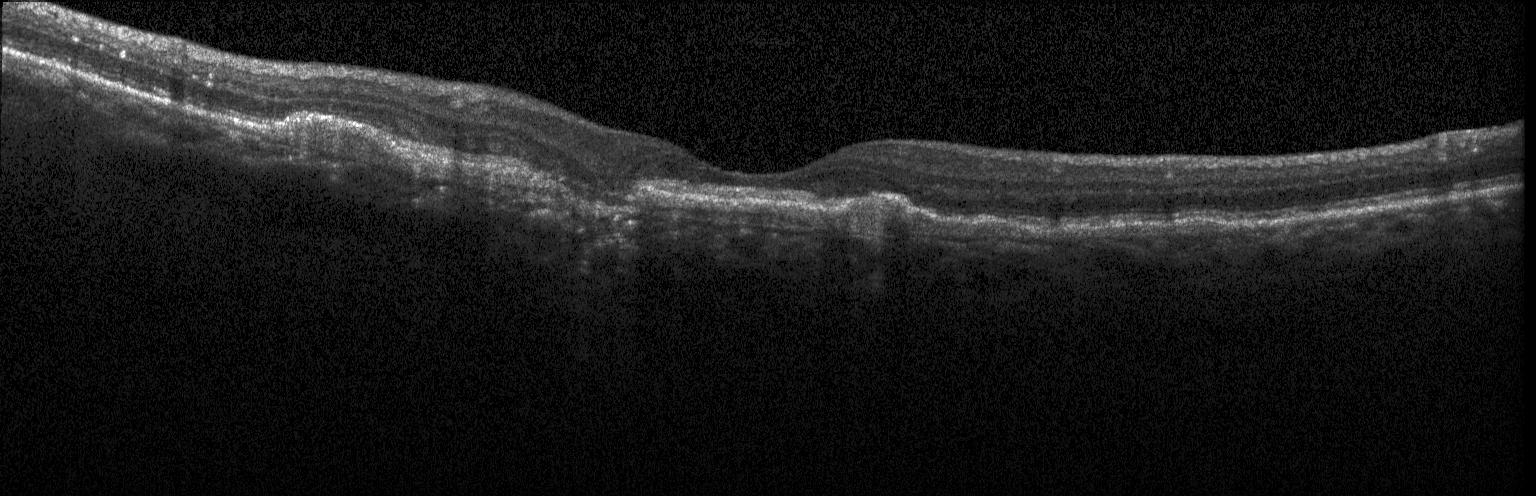

Macular OCT: choroidal neovascularization.